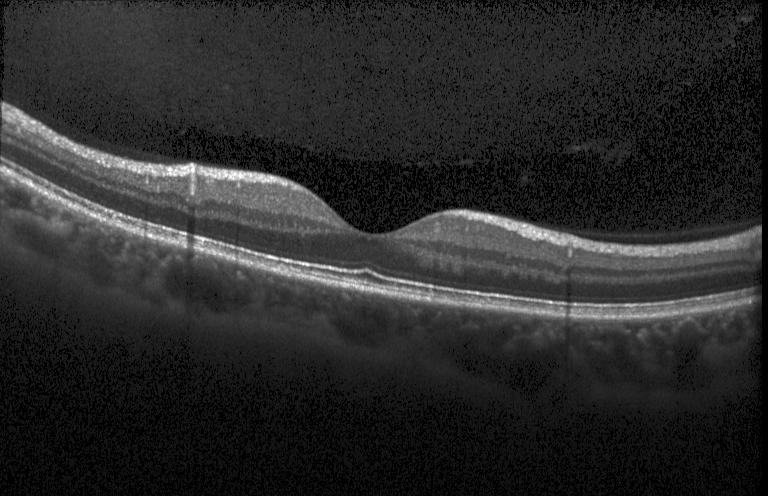 Fovea-centered, retinal OCT cross-section. This B-scan demonstrates no evidence of choroidal neovascularization, diabetic macular edema, or drusen.